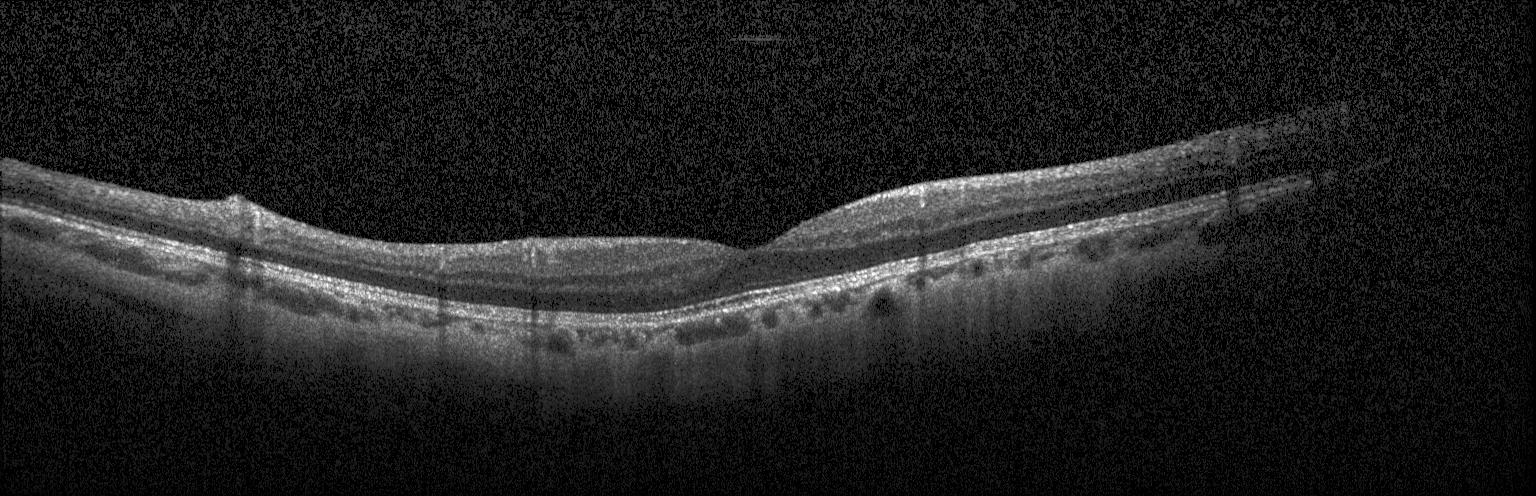
OCT line scan; acquired on a Heidelberg Spectralis; SD-OCT. Diagnosis: no evidence of choroidal neovascularization, diabetic macular edema, or drusen.